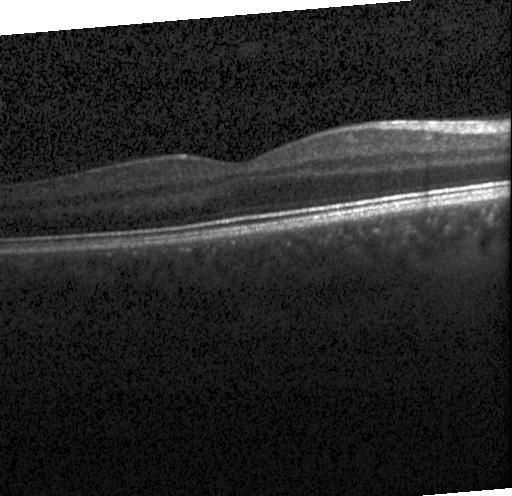
Retinal OCT B-scan, SD-OCT, instrument: Heidelberg Spectralis — No choroidal neovascularization, no diabetic macular edema, and no drusen.